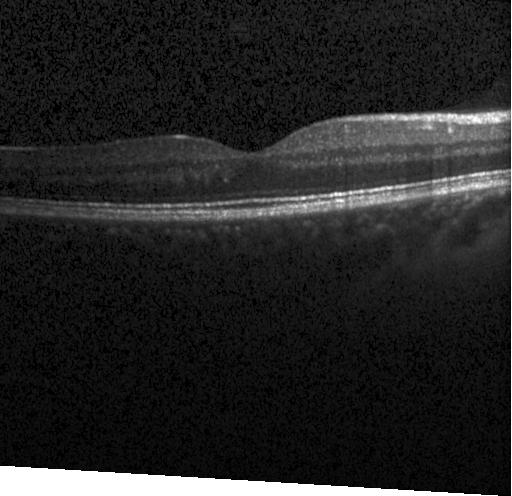 This B-scan demonstrates no choroidal neovascularization, no diabetic macular edema, and no drusen.